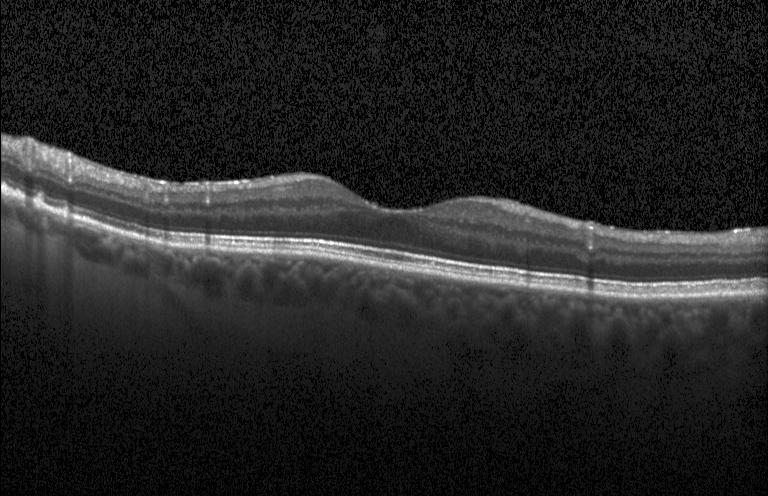
Assessment: neither choroidal neovascularization, diabetic macular edema, nor drusen.